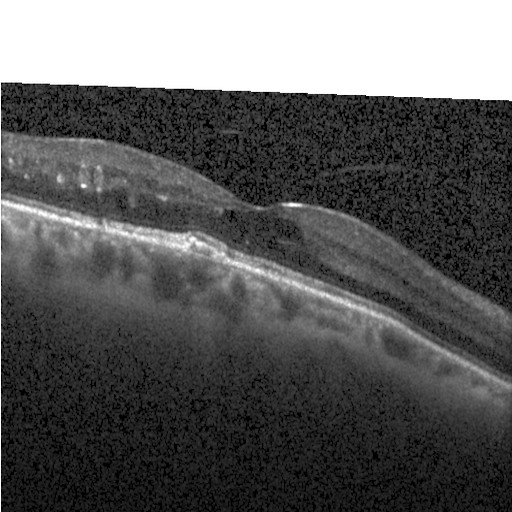

Retinal OCT B-scan · through the macula · Heidelberg Spectralis — Diagnosis: DME.